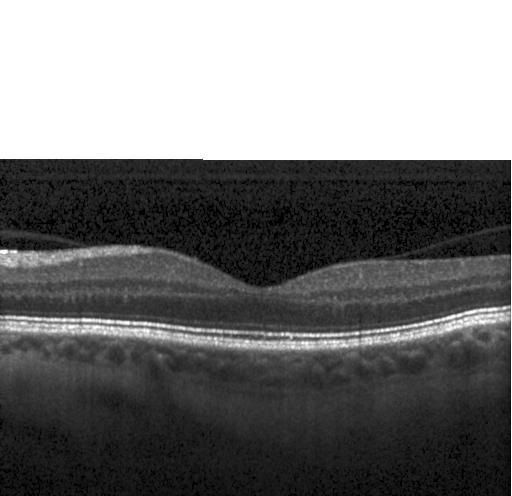 Retinal OCT cross-section, fovea-centered, Heidelberg Spectralis OCT system.
Finding: no evidence of choroidal neovascularization, diabetic macular edema, or drusen.